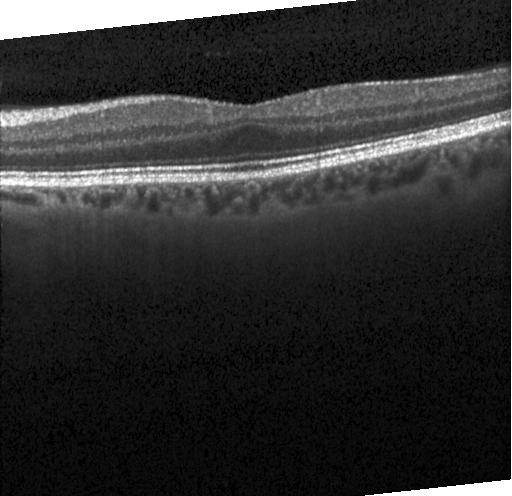
Retinal OCT cross-section — Neither CNV, DME, nor drusen.